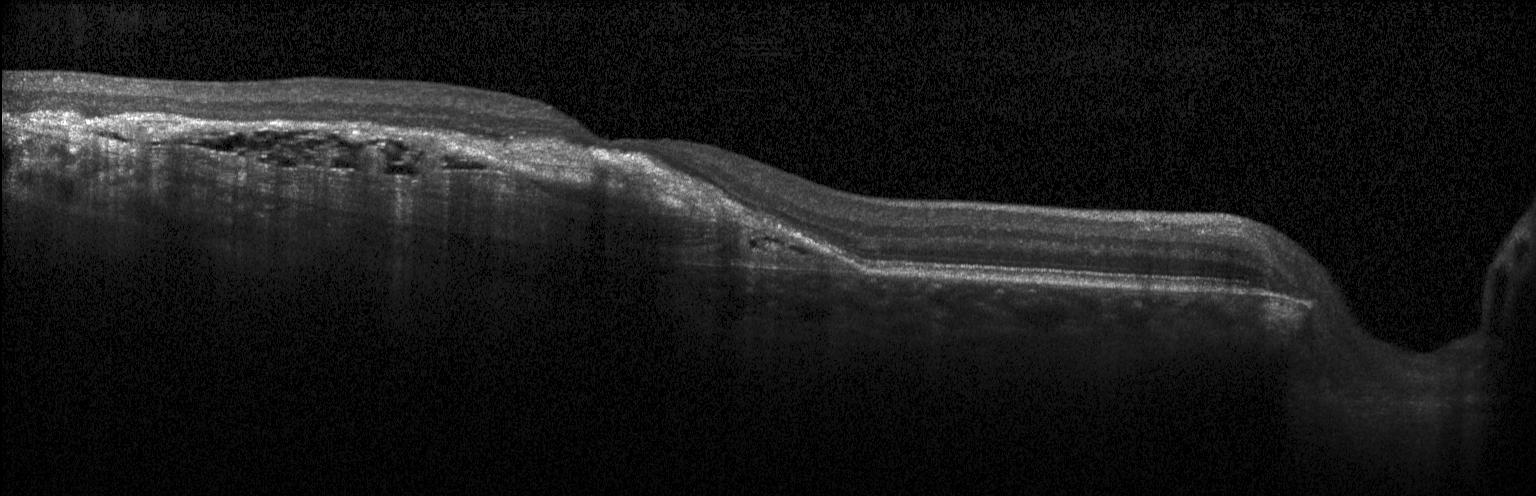

Instrument: Heidelberg Spectralis; optical coherence tomography B-scan; through the macula.
Choroidal neovascularization (CNV).